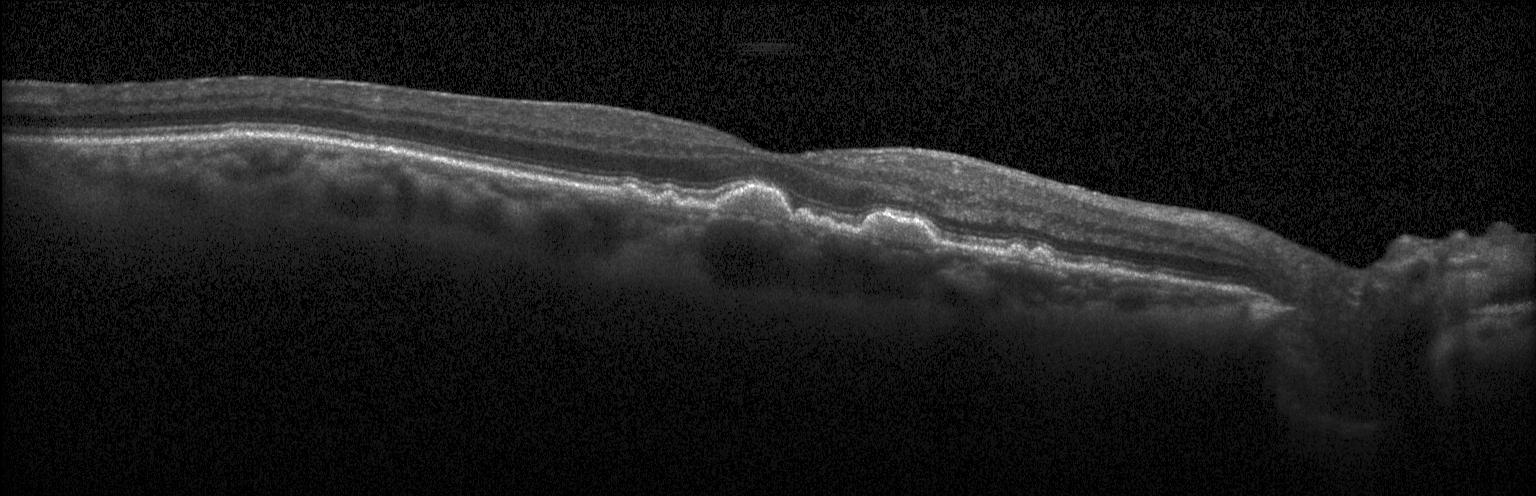 Heidelberg Spectralis · retinal OCT B-scan · spectral-domain OCT · centered on the fovea. Sub-RPE drusenoid deposits.